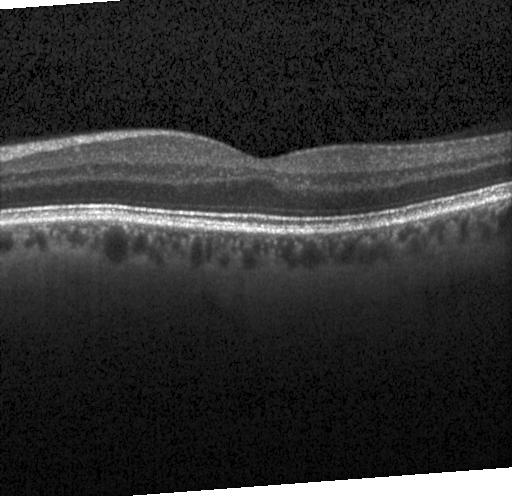 Fovea-centered. Spectral-domain optical coherence tomography. Instrument: Heidelberg Spectralis. OCT B-scan — Macular OCT: neither choroidal neovascularization, diabetic macular edema, nor drusen.